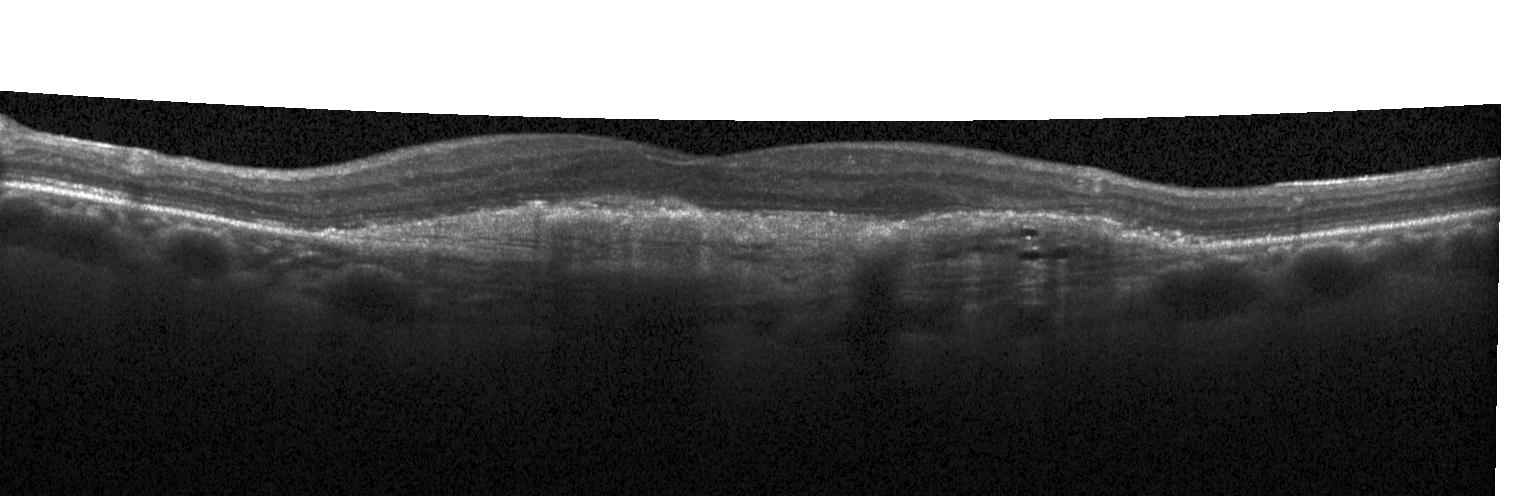 Heidelberg Spectralis · retinal OCT B-scan
Macular OCT: choroidal neovascularization.